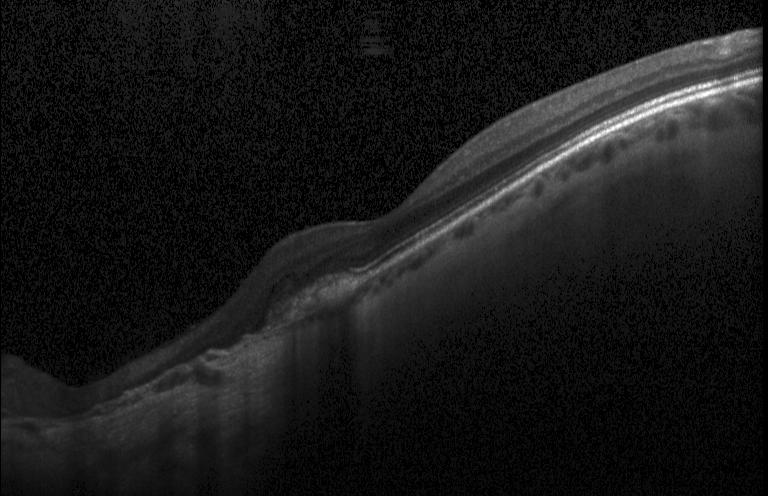 OCT line scan. Diagnosis: choroidal neovascularization (CNV).